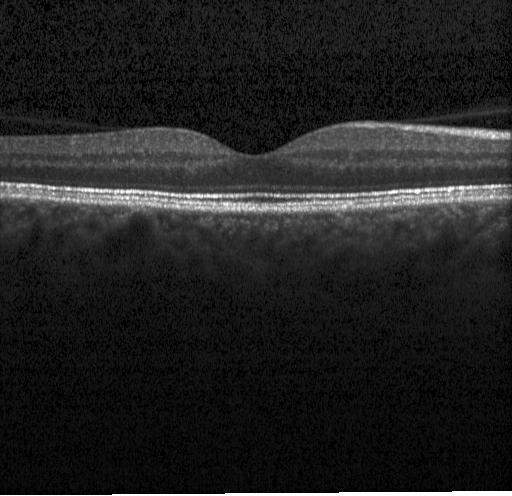 OCT line scan. OCT finding: no CNV, no DME, and no drusen.